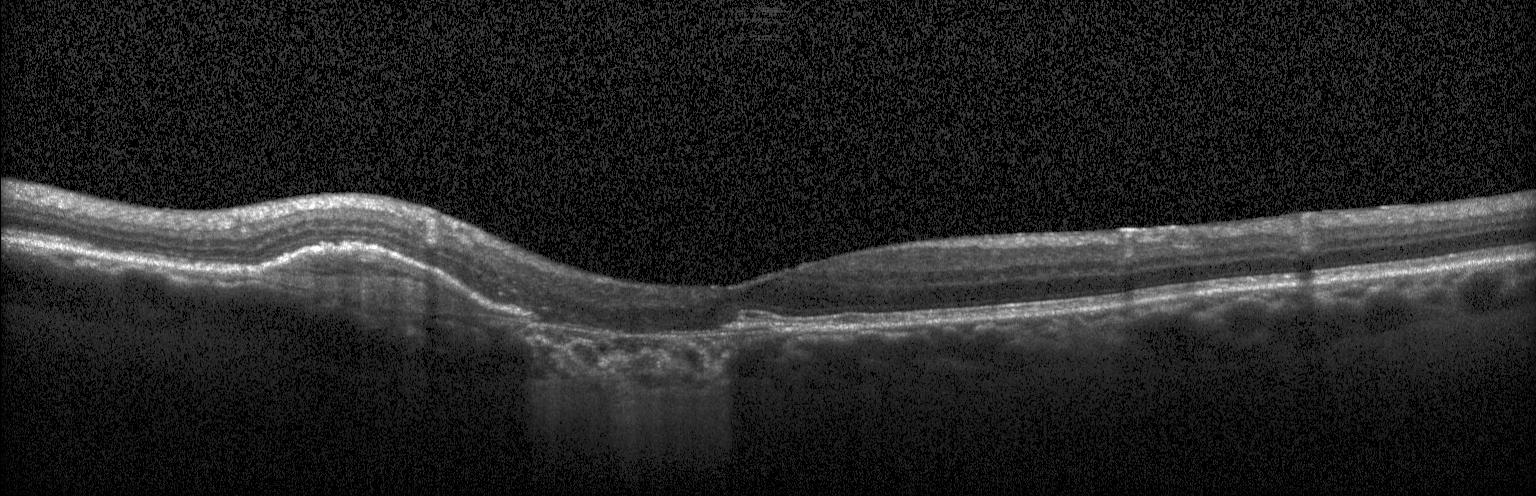 Retinal OCT cross-section, fovea-centered, instrument: Heidelberg Spectralis.
Assessment: a choroidal neovascular membrane.